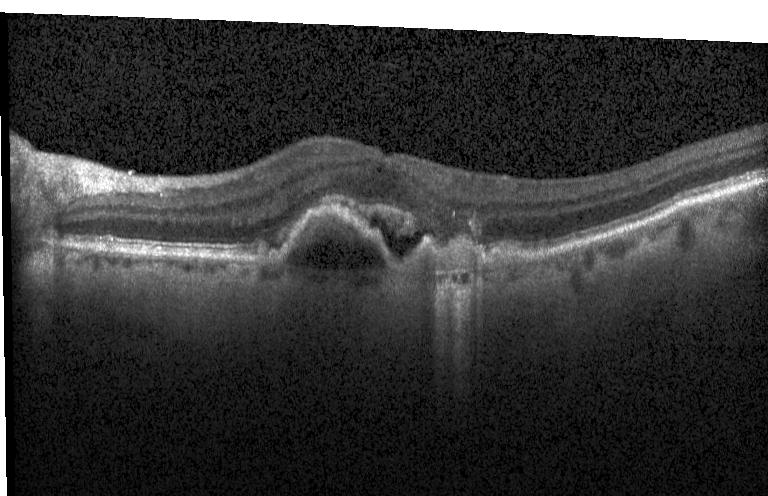 Impression: a choroidal neovascular membrane.